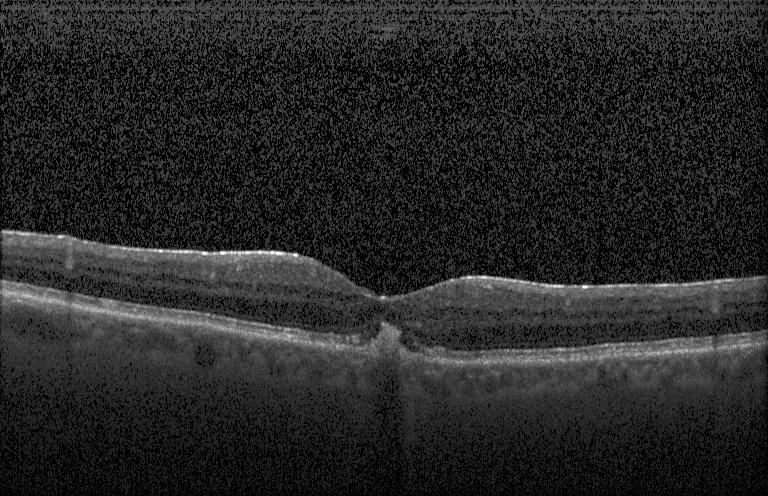 Optical coherence tomography scan · horizontal scan through the fovea · instrument: Heidelberg Spectralis — OCT finding: choroidal neovascularization (CNV).